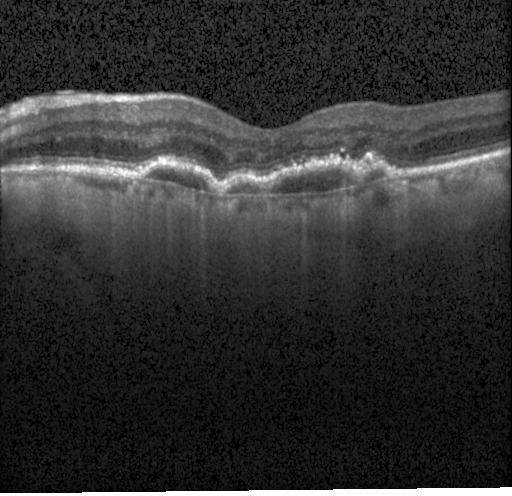 Spectral-domain OCT. OCT line scan
Dx: a choroidal neovascular membrane.